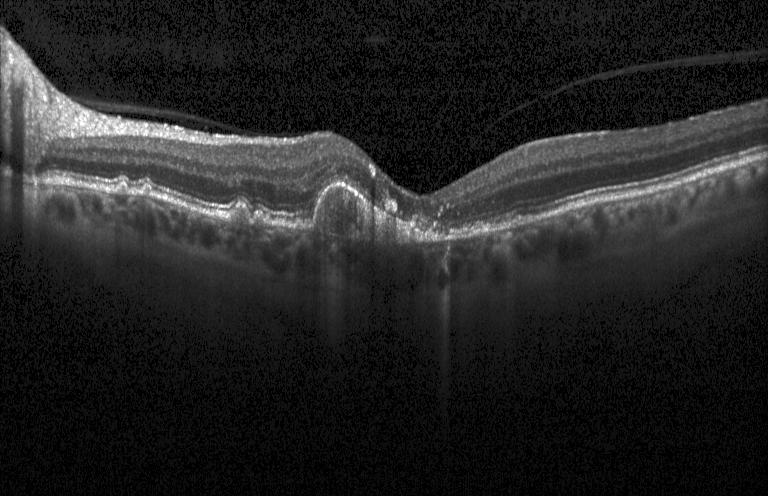
OCT B-scan; Heidelberg Spectralis OCT system; through the macula
Dx: a choroidal neovascular membrane.